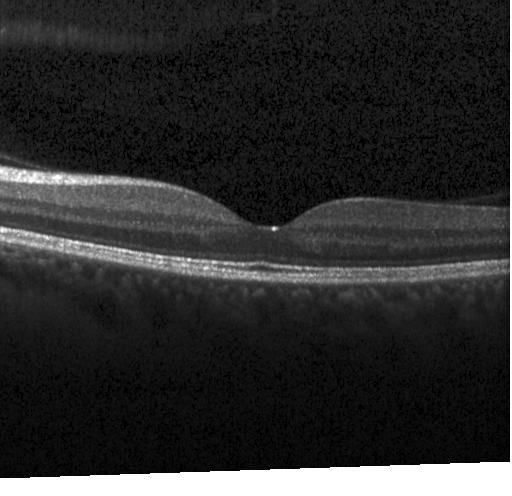 Spectral-domain OCT · OCT B-scan
Finding: neither CNV, DME, nor drusen.